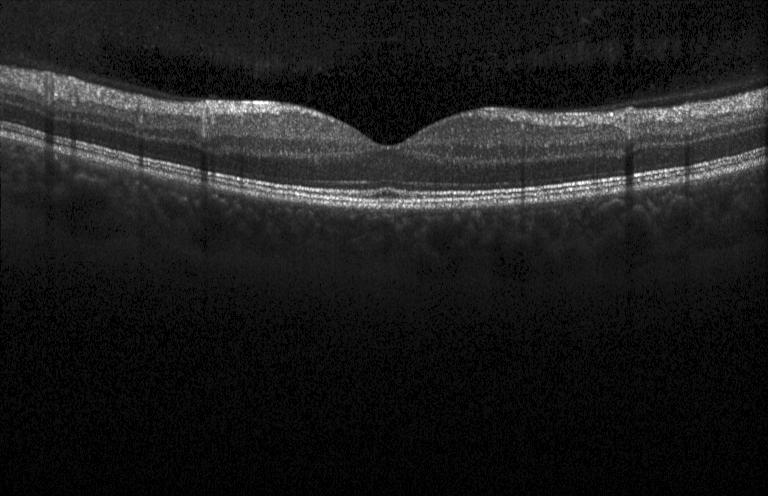 Heidelberg Spectralis OCT system · retinal OCT B-scan.
OCT finding: no evidence of CNV, DME, or drusen.